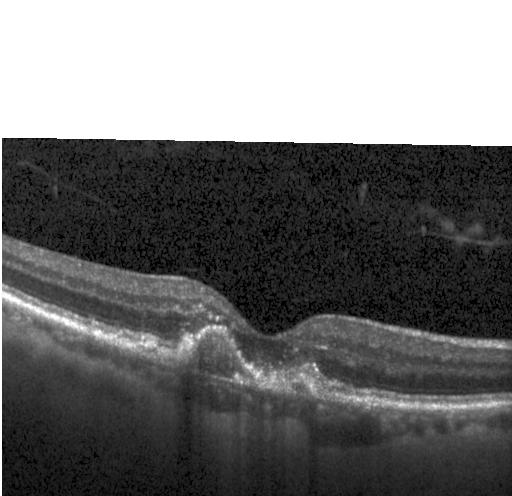
OCT B-scan showing a choroidal neovascular membrane.